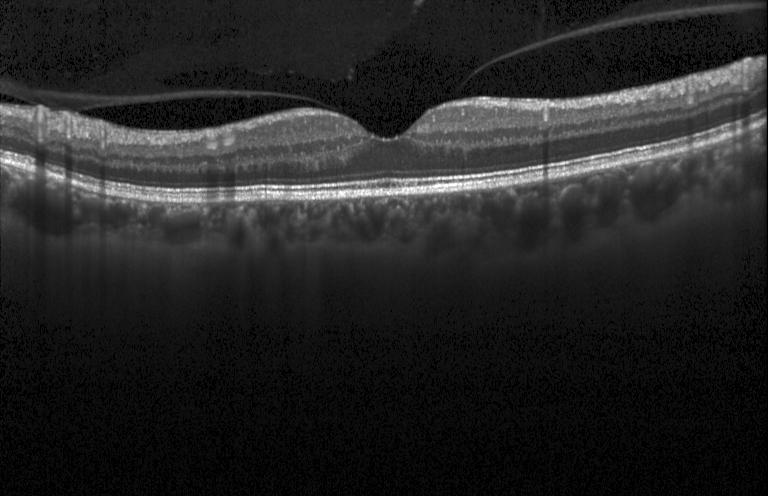

Optical coherence tomography B-scan — Diagnosis: no evidence of choroidal neovascularization, diabetic macular edema, or drusen.